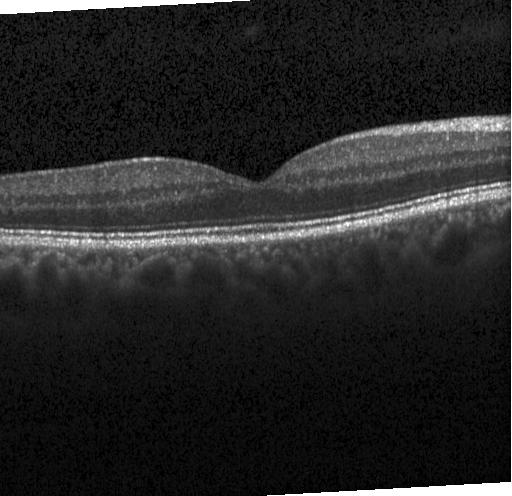

Retinal OCT cross-section — Diagnosis: no choroidal neovascularization, diabetic macular edema, or drusen.